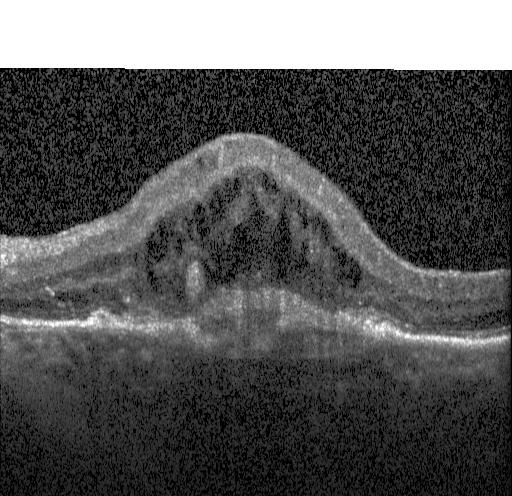 Spectral-domain OCT; acquired on a Heidelberg Spectralis; OCT line scan; fovea-centered
Finding: CNV.